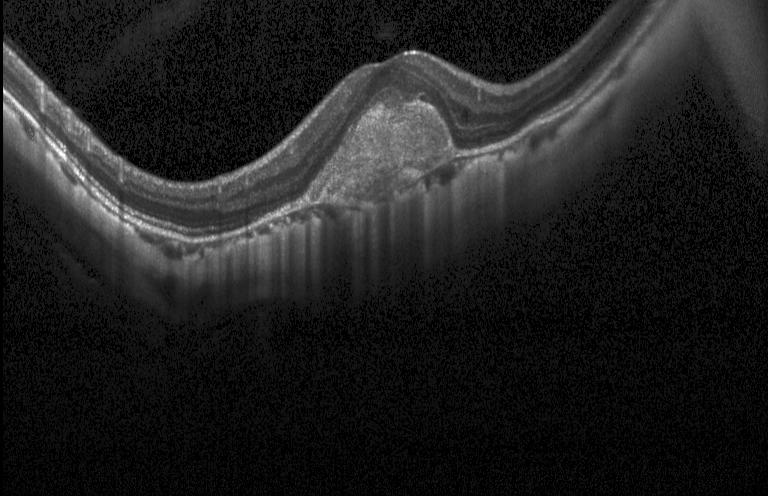 The scan shows a choroidal neovascular membrane.